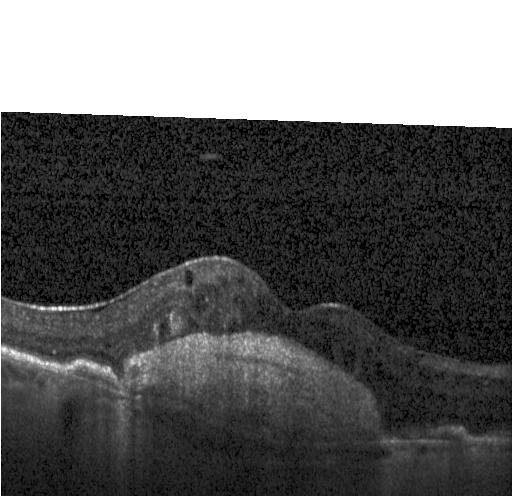 Impression: a choroidal neovascular membrane.